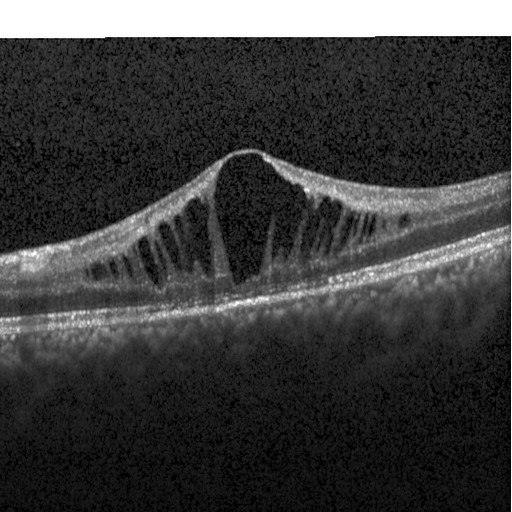
Macular scan. Optical coherence tomography B-scan. Spectral-domain optical coherence tomography.
Finding: DME.